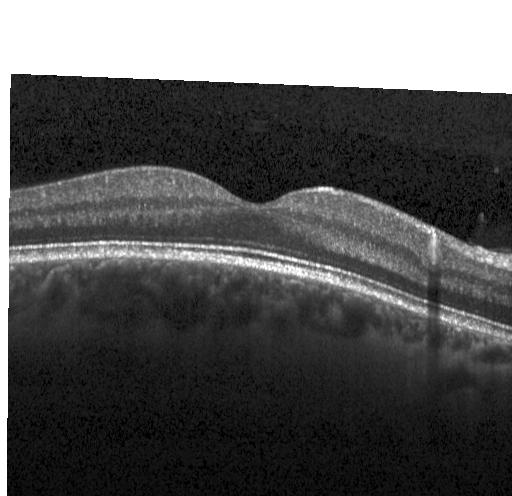 OCT B-scan showing neither CNV, DME, nor drusen.